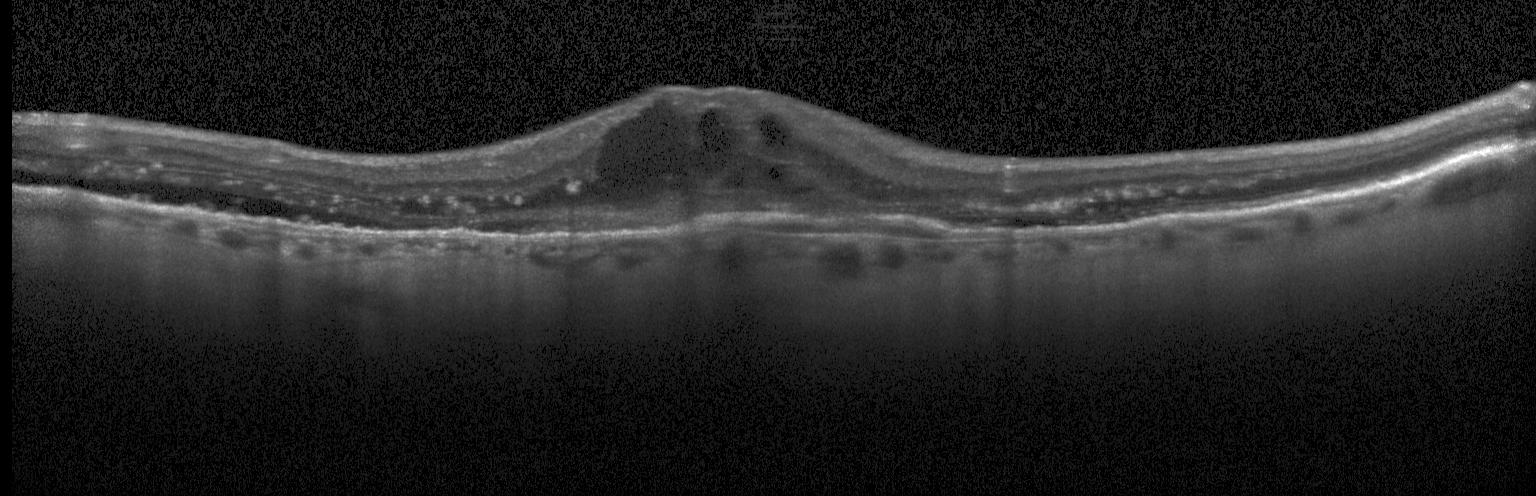

Choroidal neovascularization.